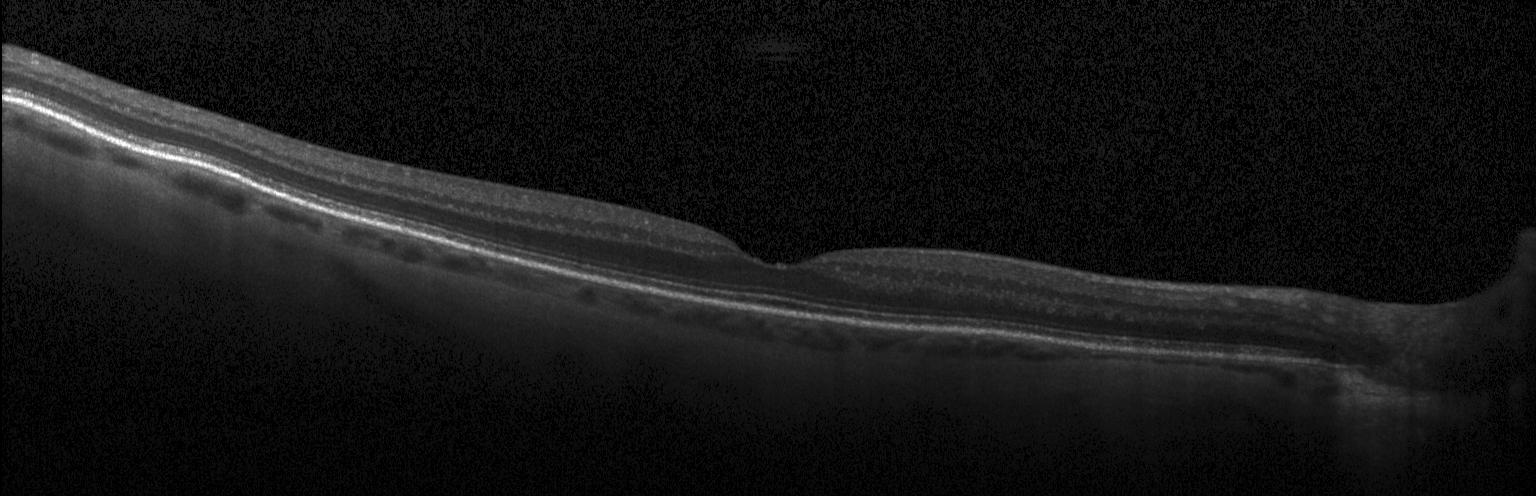
Dx: no choroidal neovascularization, no diabetic macular edema, and no drusen.